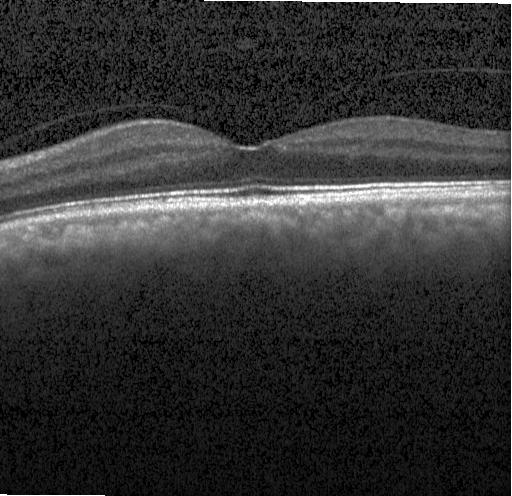
Impression: no CNV, DME, or drusen.